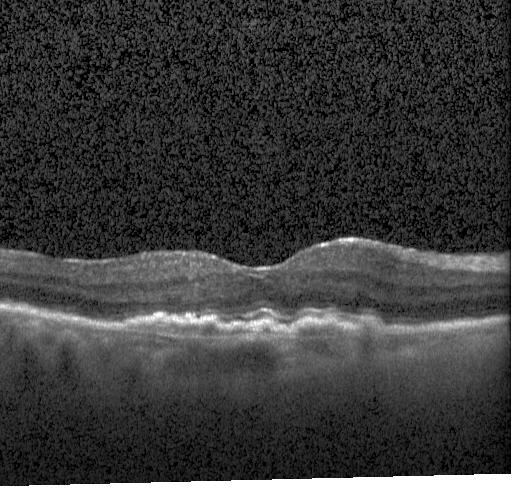

Macular OCT: CNV.